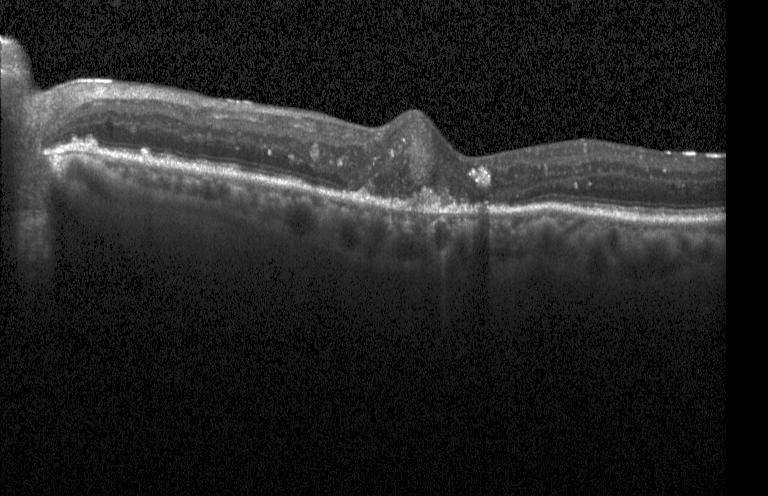
Heidelberg Spectralis, SD-OCT, optical coherence tomography scan, macular scan. Finding: choroidal neovascularization (CNV).